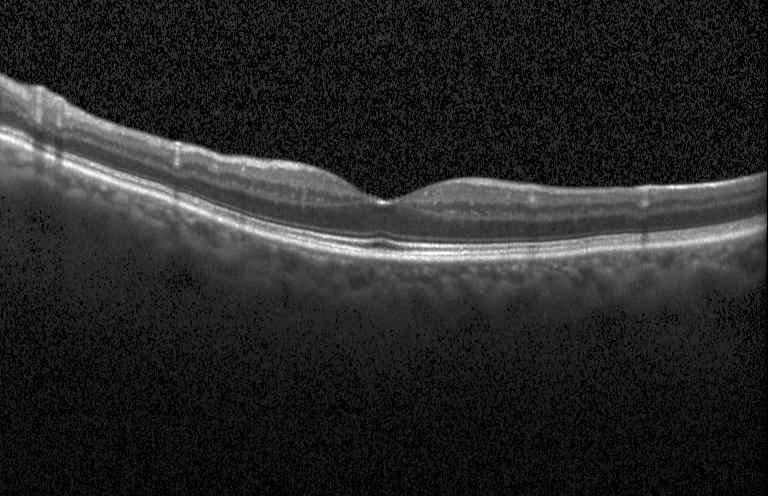

Diagnosis: no choroidal neovascularization, no diabetic macular edema, and no drusen.